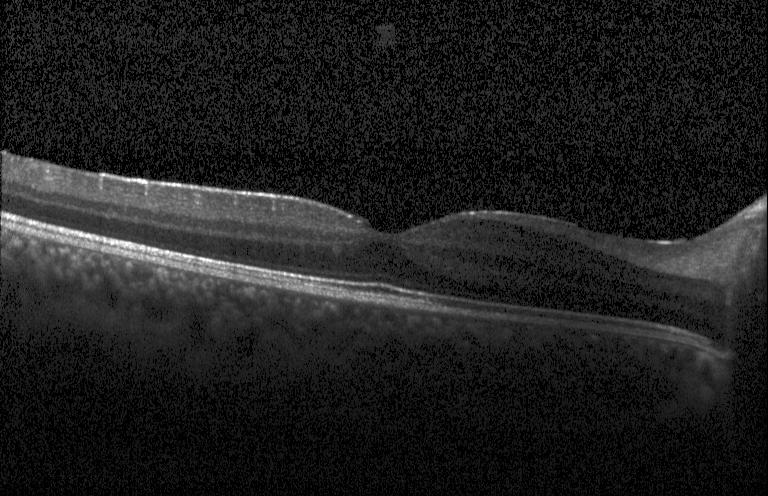 OCT B-scan showing neither choroidal neovascularization, diabetic macular edema, nor drusen.